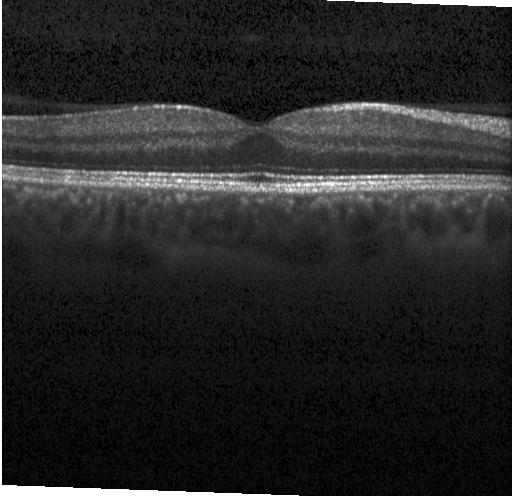 Retinal OCT cross-section — Dx: neither choroidal neovascularization, diabetic macular edema, nor drusen.